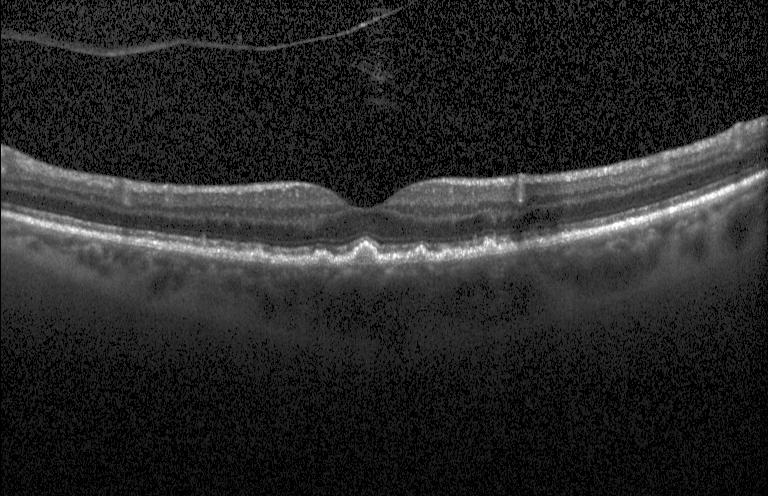 Retinal OCT cross-section, SD-OCT
This B-scan demonstrates multiple drusen.